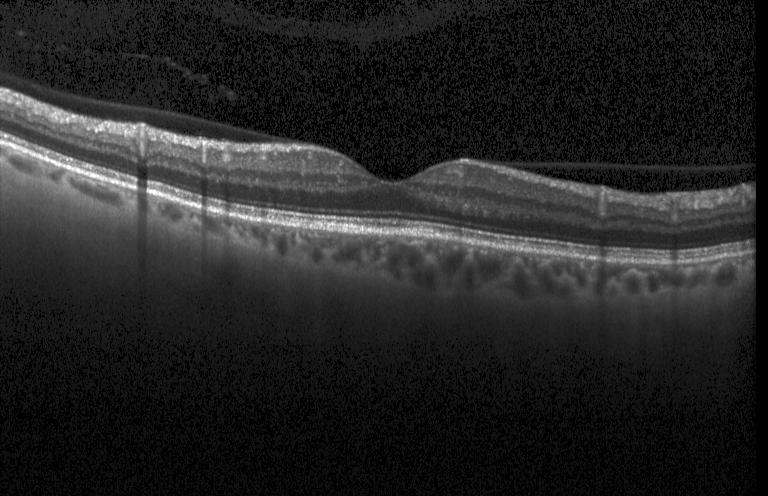

OCT line scan, instrument: Heidelberg Spectralis, spectral-domain optical coherence tomography — This B-scan demonstrates no evidence of CNV, DME, or drusen.